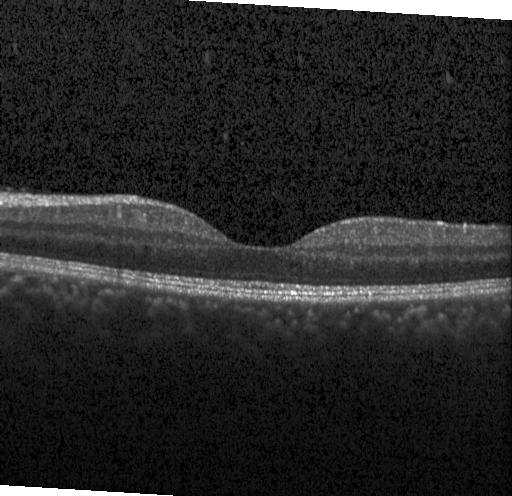 Retinal OCT cross-section showing no choroidal neovascularization, no diabetic macular edema, and no drusen.